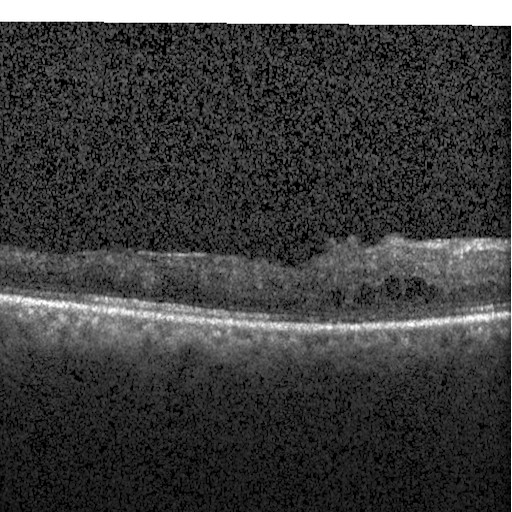
Macular OCT demonstrating diabetic macular edema (DME).